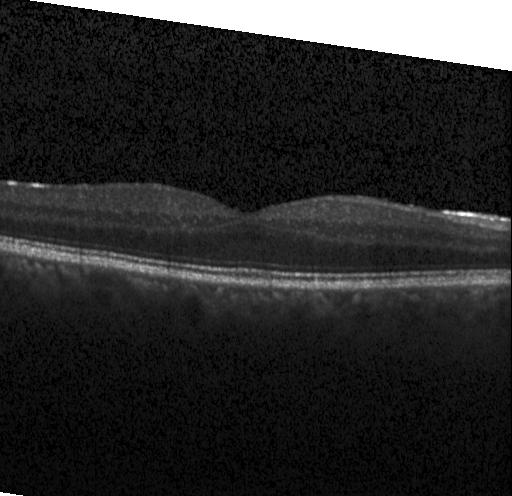 Centered on the fovea. Spectral-domain OCT. OCT line scan. Instrument: Heidelberg Spectralis. Assessment: no CNV, no DME, and no drusen.